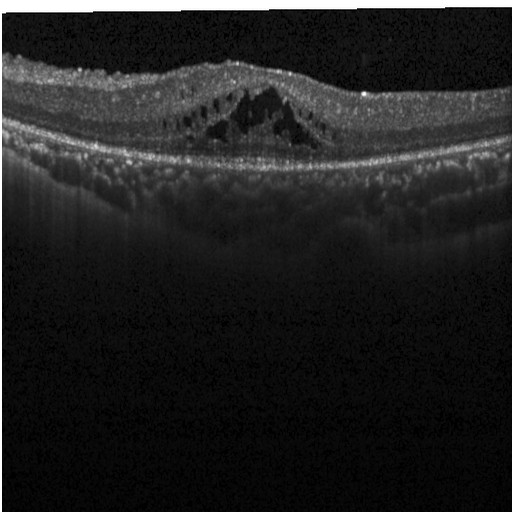

Diagnosis: DME.